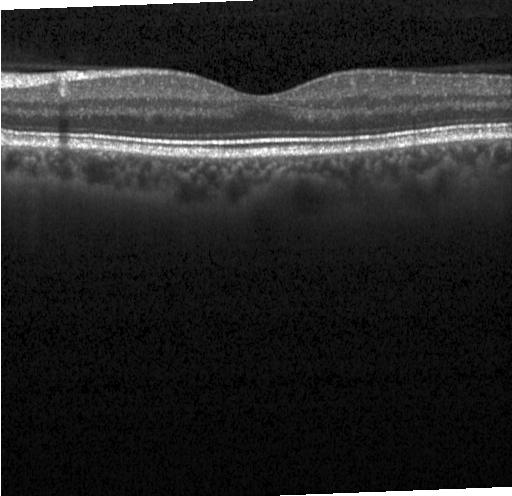
Fovea-centered; retinal OCT cross-section; Heidelberg Spectralis OCT system; spectral-domain optical coherence tomography. Impression: neither choroidal neovascularization, diabetic macular edema, nor drusen.